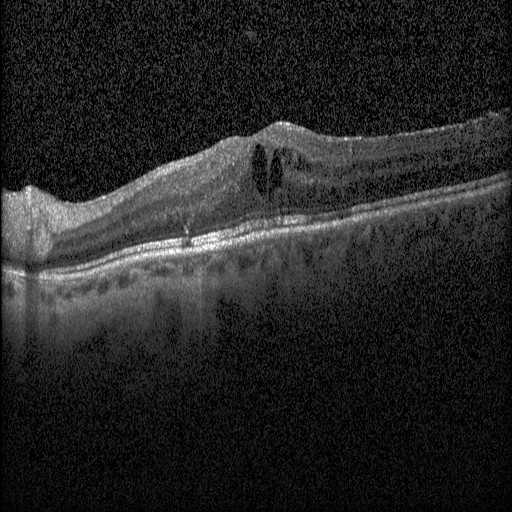 OCT line scan. Assessment: diabetic macular edema.